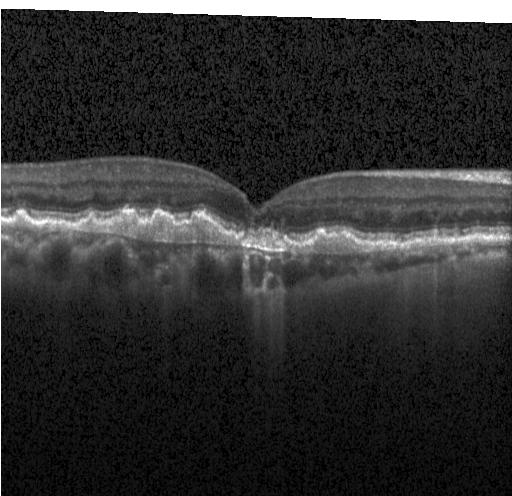 OCT scan showing a choroidal neovascular membrane.